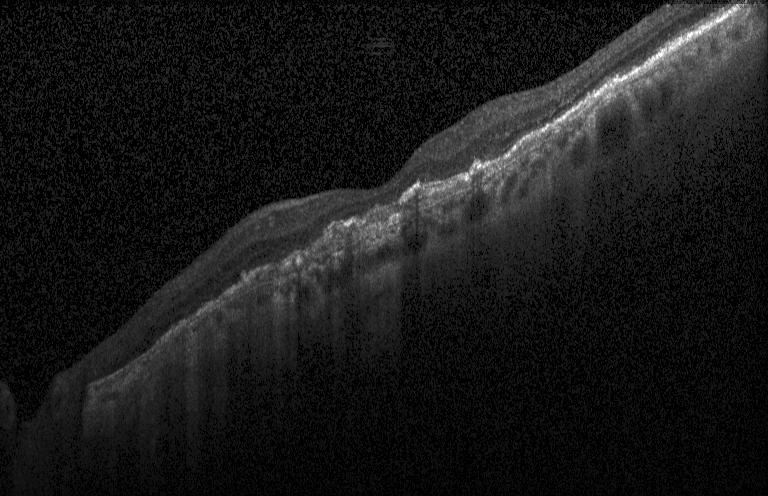
Acquired on a Heidelberg Spectralis, OCT line scan, centered on the fovea — Diagnosis: choroidal neovascularization (CNV).